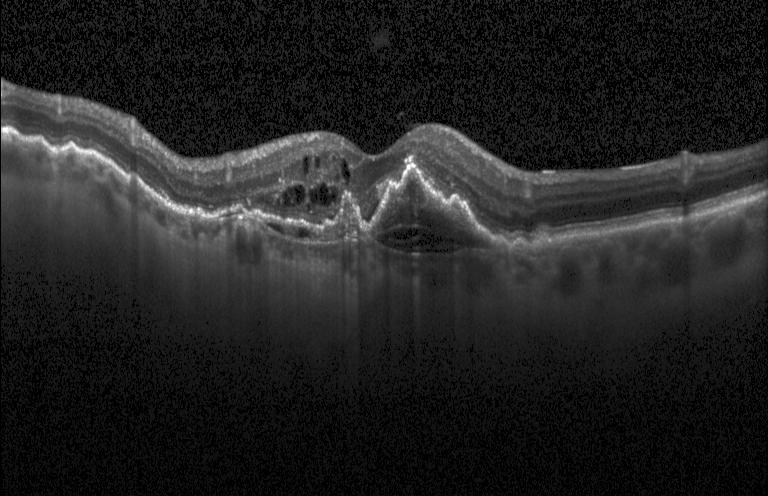

Retinal OCT B-scan; acquired on a Heidelberg Spectralis.
Dx: a choroidal neovascular membrane.